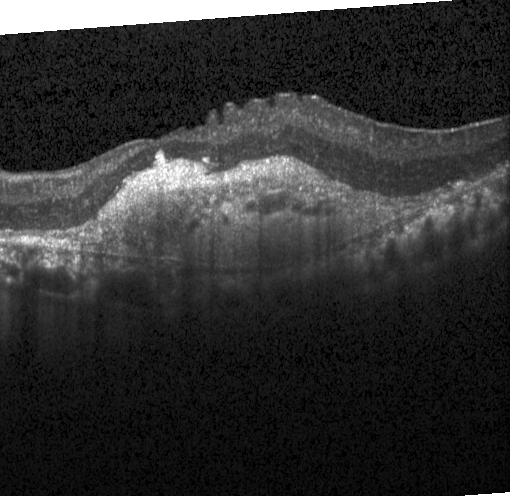
OCT B-scan — Finding: a choroidal neovascular membrane.